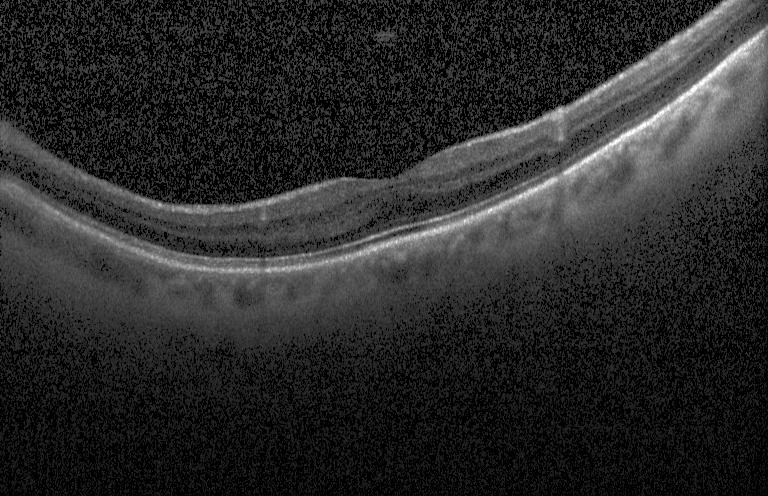
Acquired on a Heidelberg Spectralis; through the macula; retinal OCT cross-section.
Diagnosis: neither choroidal neovascularization, diabetic macular edema, nor drusen.